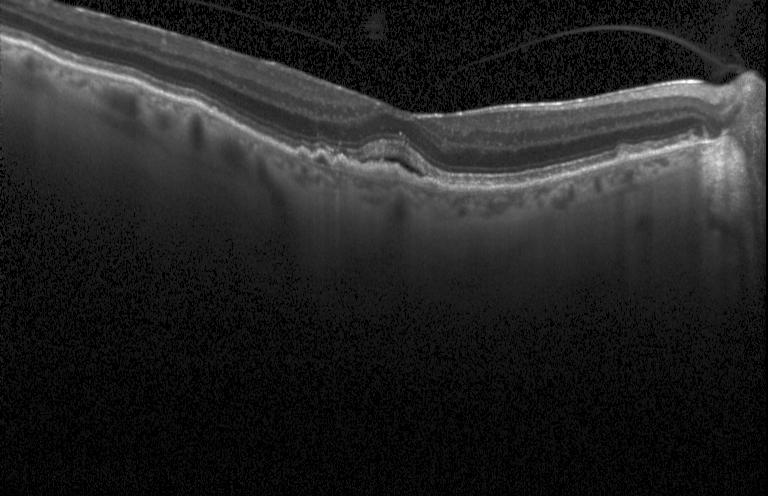 Spectral-domain optical coherence tomography, through the macula, optical coherence tomography B-scan, Heidelberg Spectralis — Dx: choroidal neovascularization.